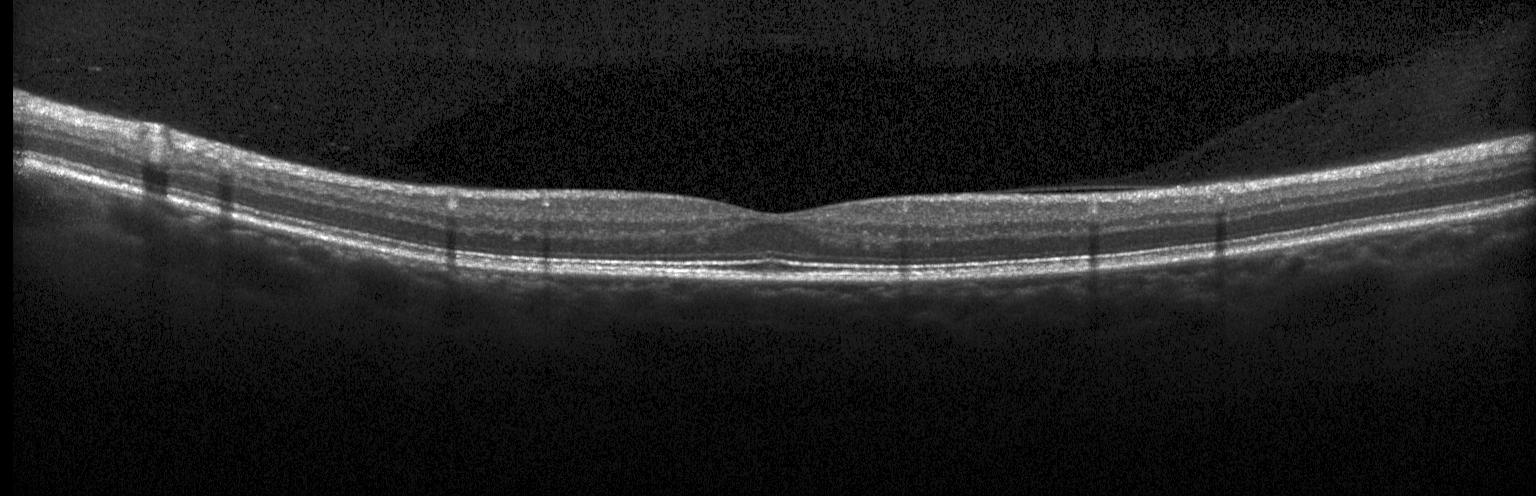

Finding: no CNV, no DME, and no drusen.